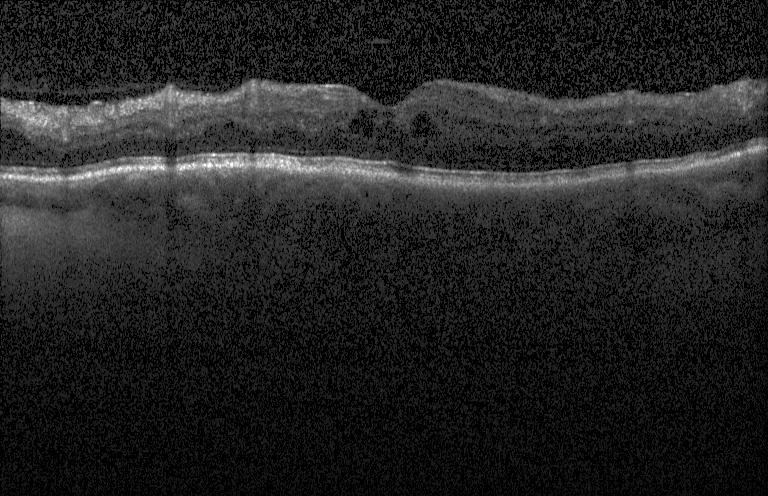
Macular scan. Spectral-domain optical coherence tomography. Retinal OCT B-scan.
The scan shows diabetic macular edema.